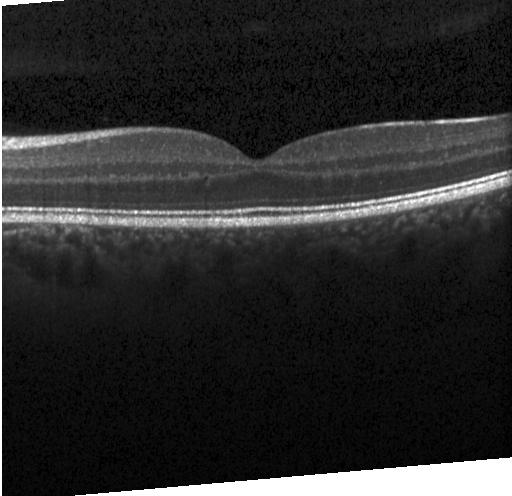

Retinal OCT cross-section showing no evidence of CNV, DME, or drusen.